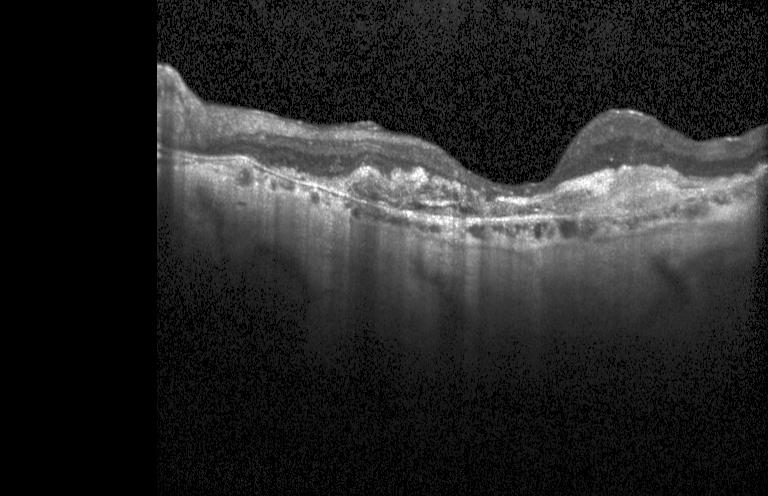 Heidelberg Spectralis OCT system; optical coherence tomography scan. OCT finding: choroidal neovascularization (CNV).